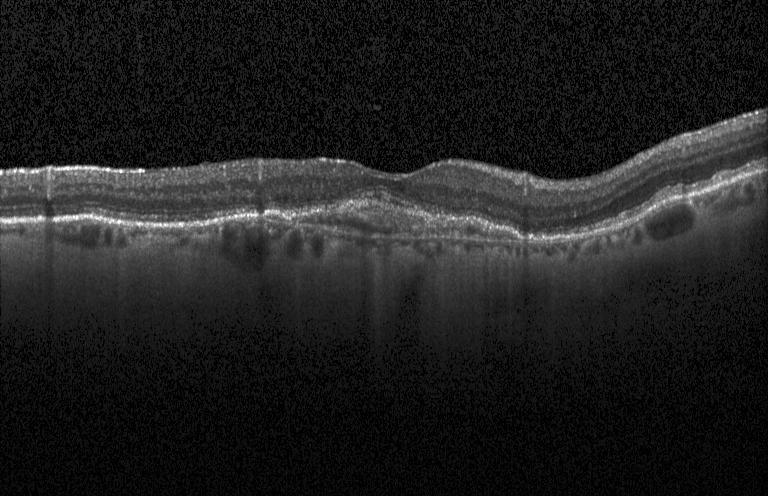 SD-OCT, Heidelberg Spectralis, retinal OCT cross-section
Impression: CNV.